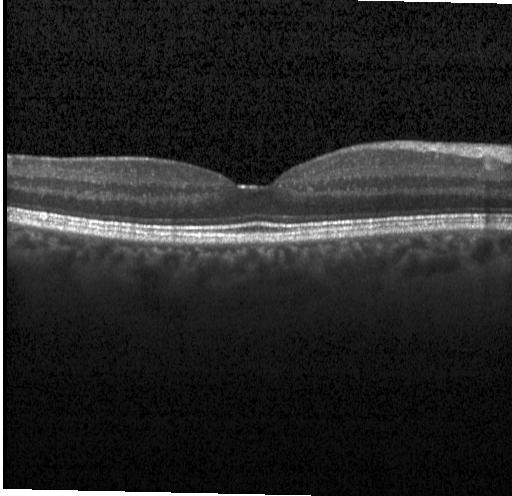

Retinal OCT B-scan.
Diagnosis: no choroidal neovascularization, diabetic macular edema, or drusen.